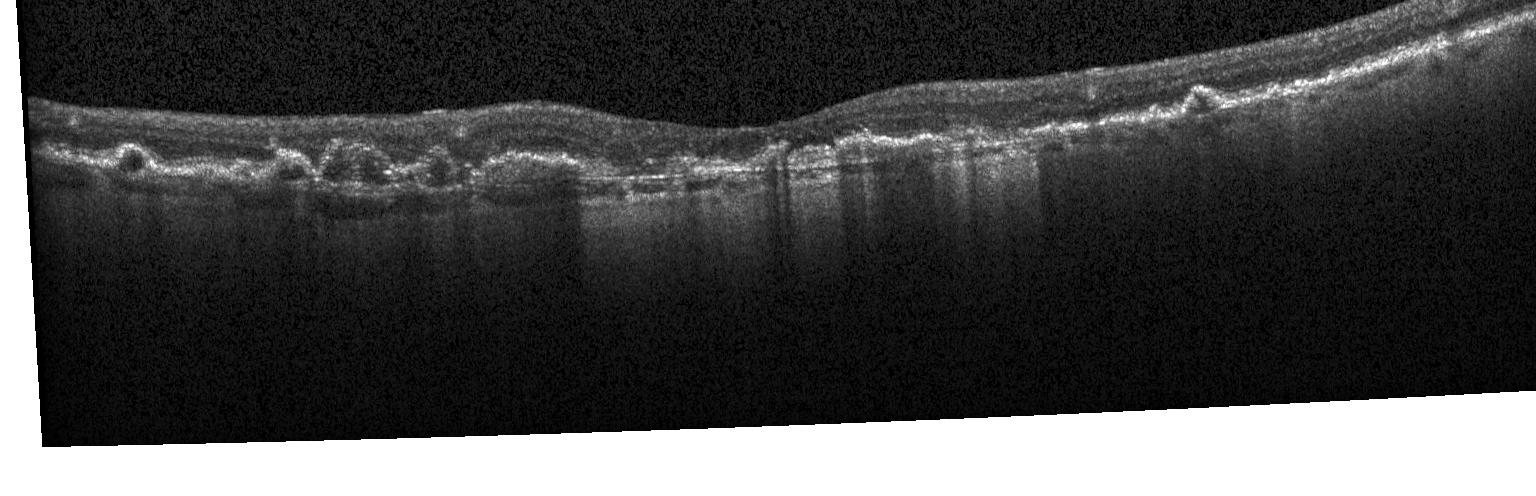

Heidelberg Spectralis; optical coherence tomography scan; spectral-domain OCT — Impression: choroidal neovascularization (CNV).